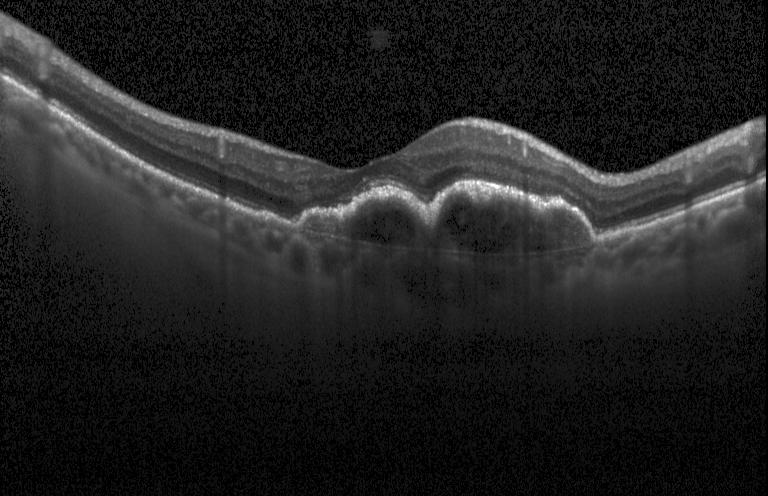

Retinal OCT B-scan · Heidelberg Spectralis OCT system. Dx: CNV.